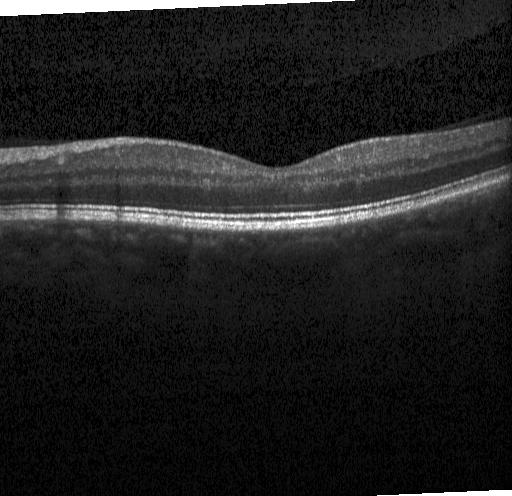
Optical coherence tomography scan.
Impression: neither CNV, DME, nor drusen.